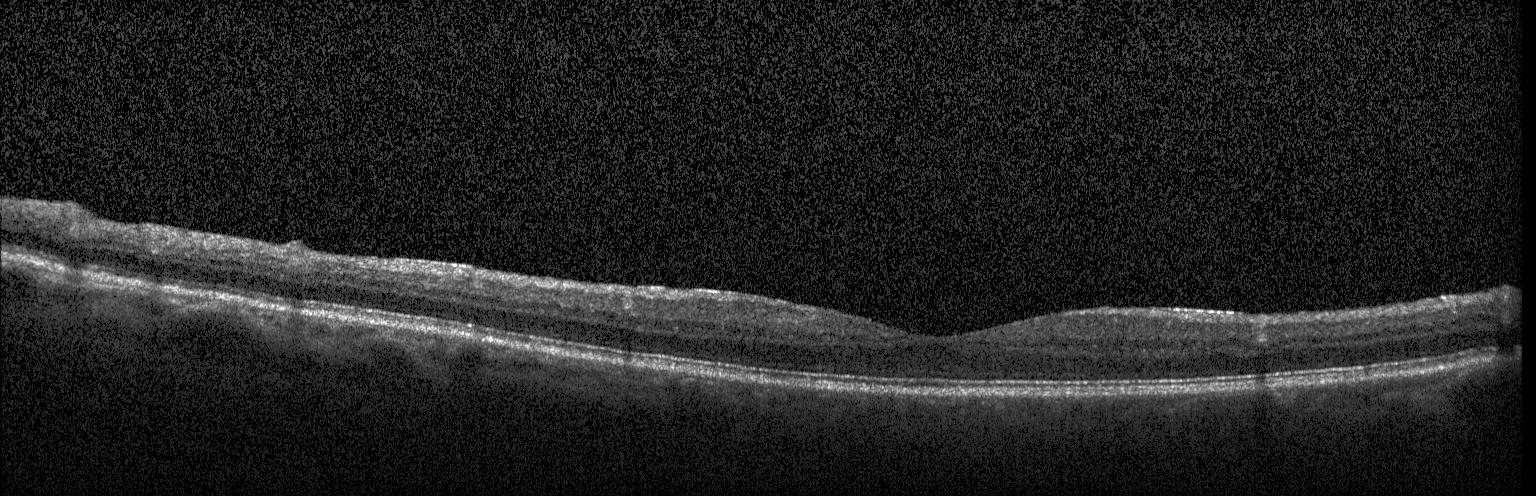

SD-OCT, retinal OCT B-scan. This B-scan demonstrates neither CNV, DME, nor drusen.